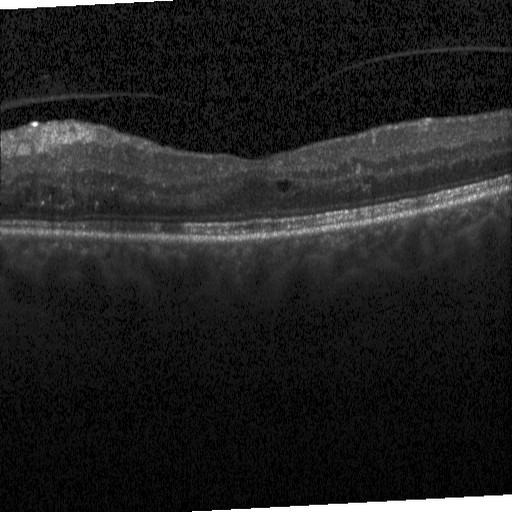
OCT scan showing diabetic macular edema (DME).